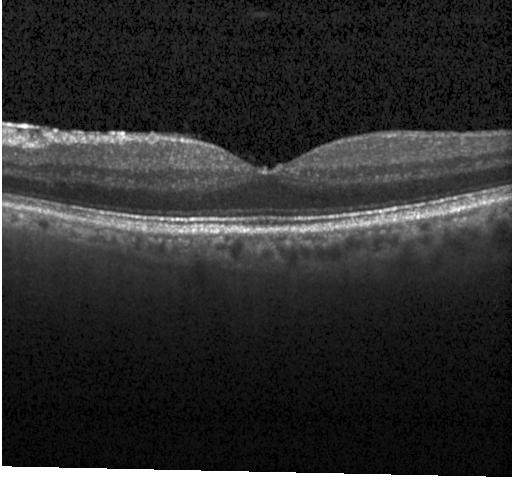
Optical coherence tomography B-scan.
Macular OCT: no choroidal neovascularization, diabetic macular edema, or drusen.